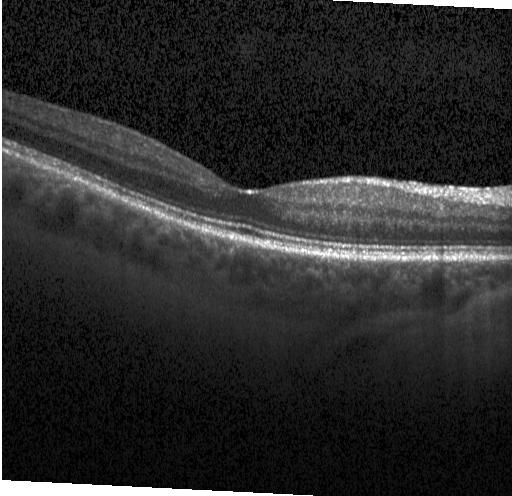 Optical coherence tomography scan; Heidelberg Spectralis OCT system; horizontal scan through the fovea
Finding: no choroidal neovascularization, no diabetic macular edema, and no drusen.